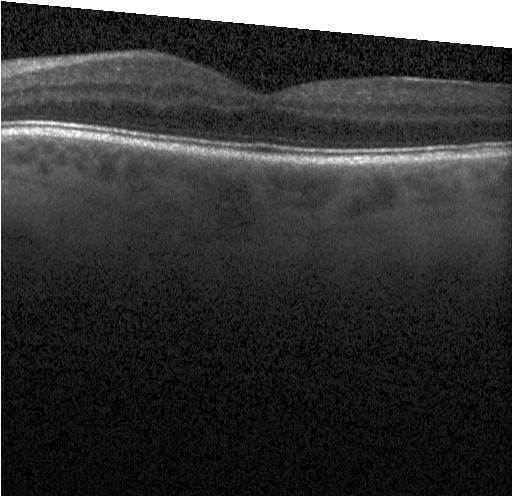 SD-OCT. Optical coherence tomography B-scan. Horizontal scan through the fovea
OCT finding: neither CNV, DME, nor drusen.